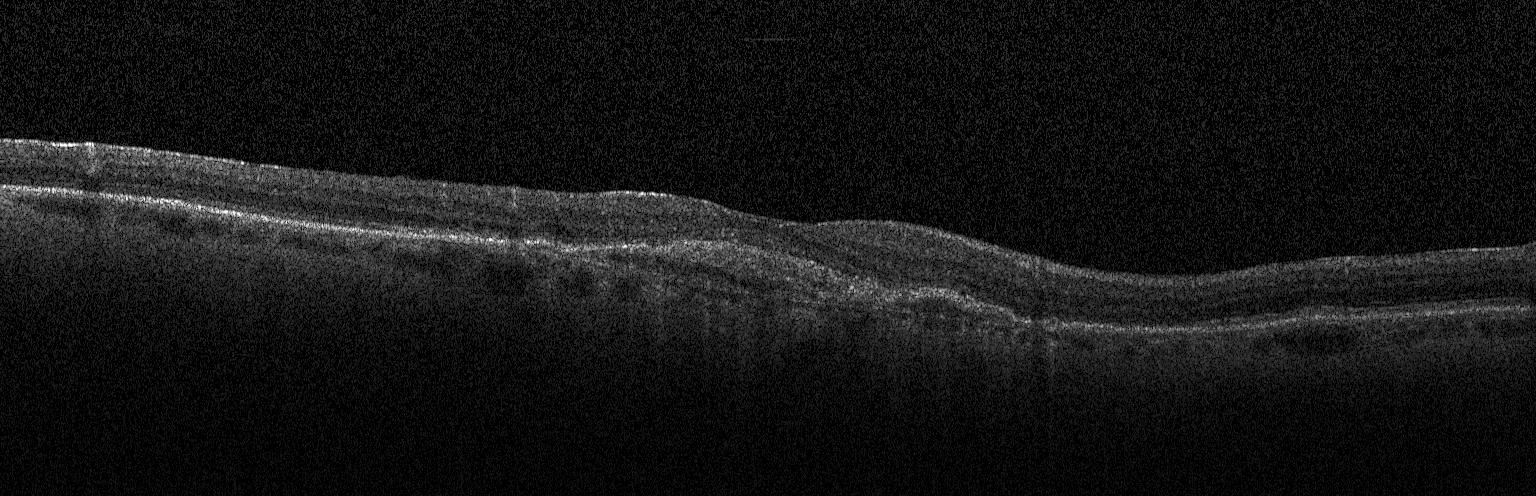
Macular OCT: choroidal neovascularization (CNV).